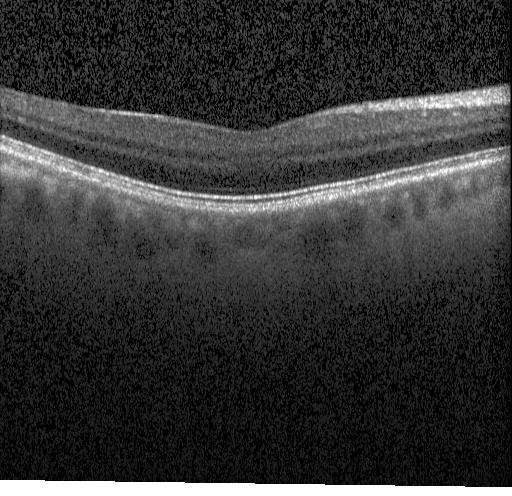

Retinal OCT B-scan, fovea-centered.
Finding: no evidence of CNV, DME, or drusen.